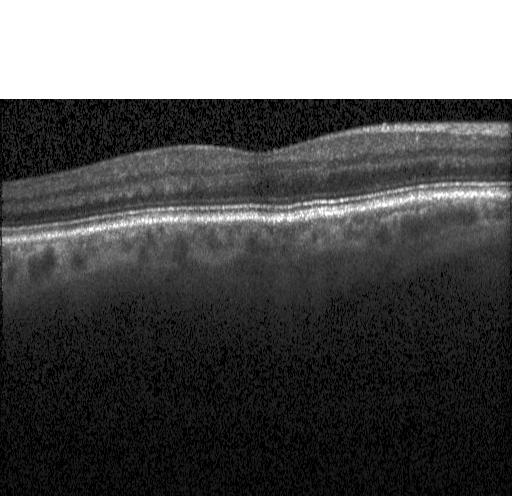

OCT B-scan
Macular OCT: neither choroidal neovascularization, diabetic macular edema, nor drusen.